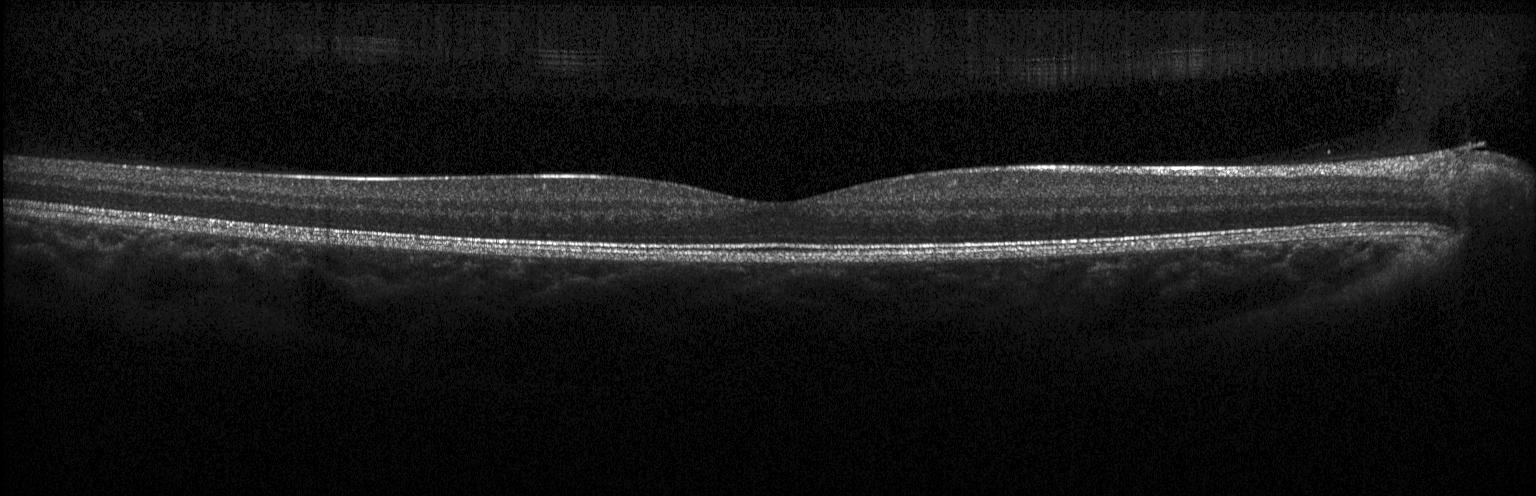
Impression: neither CNV, DME, nor drusen.